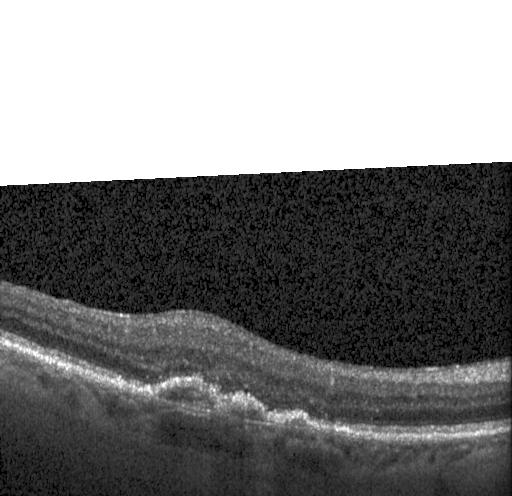 Optical coherence tomography scan — Impression: a choroidal neovascular membrane.